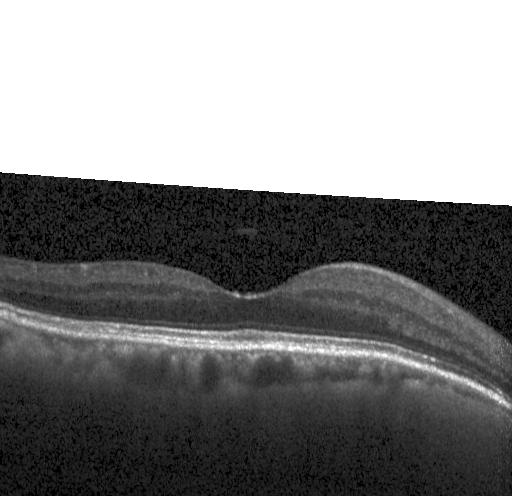

Retinal OCT B-scan
Finding: no CNV, no DME, and no drusen.